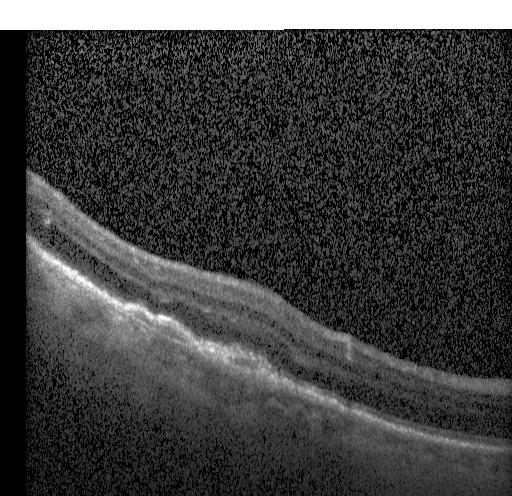

Heidelberg Spectralis OCT system · OCT B-scan. The scan shows a choroidal neovascular membrane.